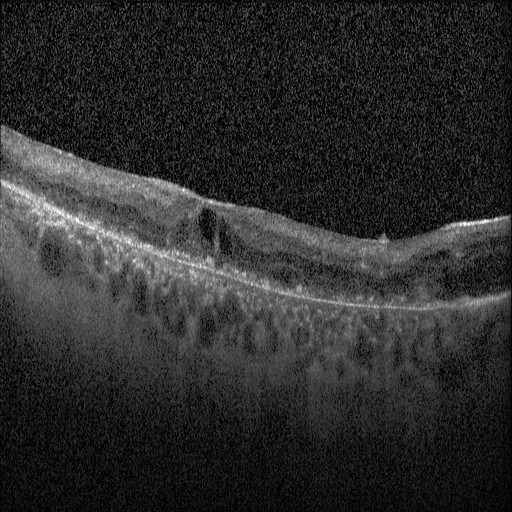
Optical coherence tomography scan; centered on the fovea
DME.